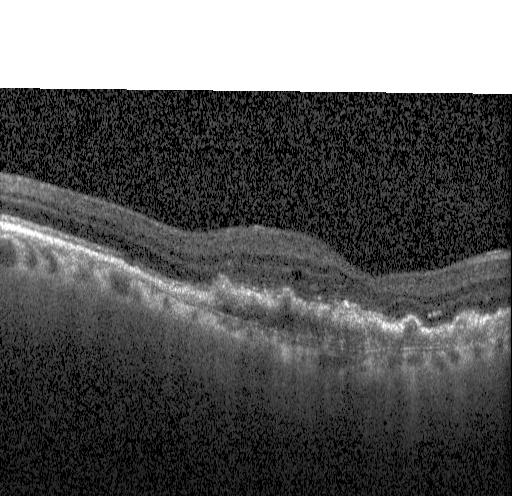 OCT B-scan · spectral-domain optical coherence tomography · fovea-centered
Assessment: a choroidal neovascular membrane.